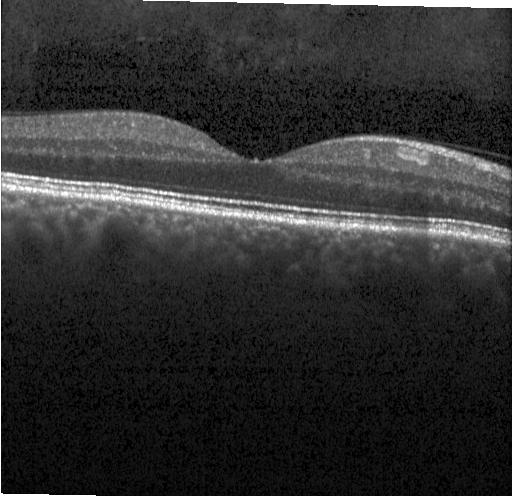

Spectral-domain OCT B-scan: no CNV, DME, or drusen.